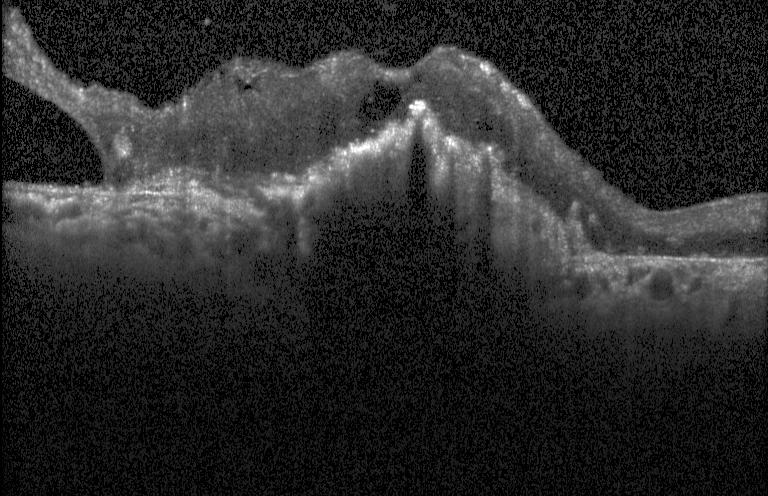
Assessment: choroidal neovascularization (CNV).